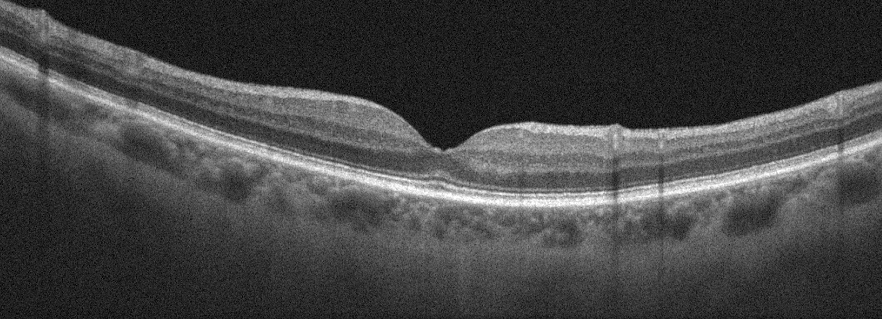
Optical coherence tomography scan, oculus dexter, macular scan — The scan shows absence of AMD, DME, ERM, RAO, RVO, and vitreomacular interface disease.